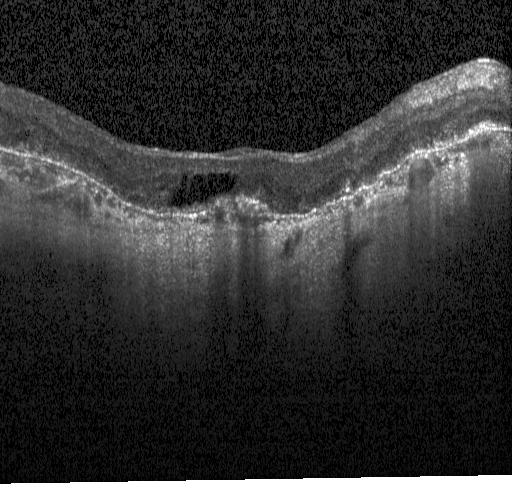
Spectral-domain optical coherence tomography · OCT line scan · through the macula · Heidelberg Spectralis OCT system. This B-scan demonstrates a choroidal neovascular membrane.